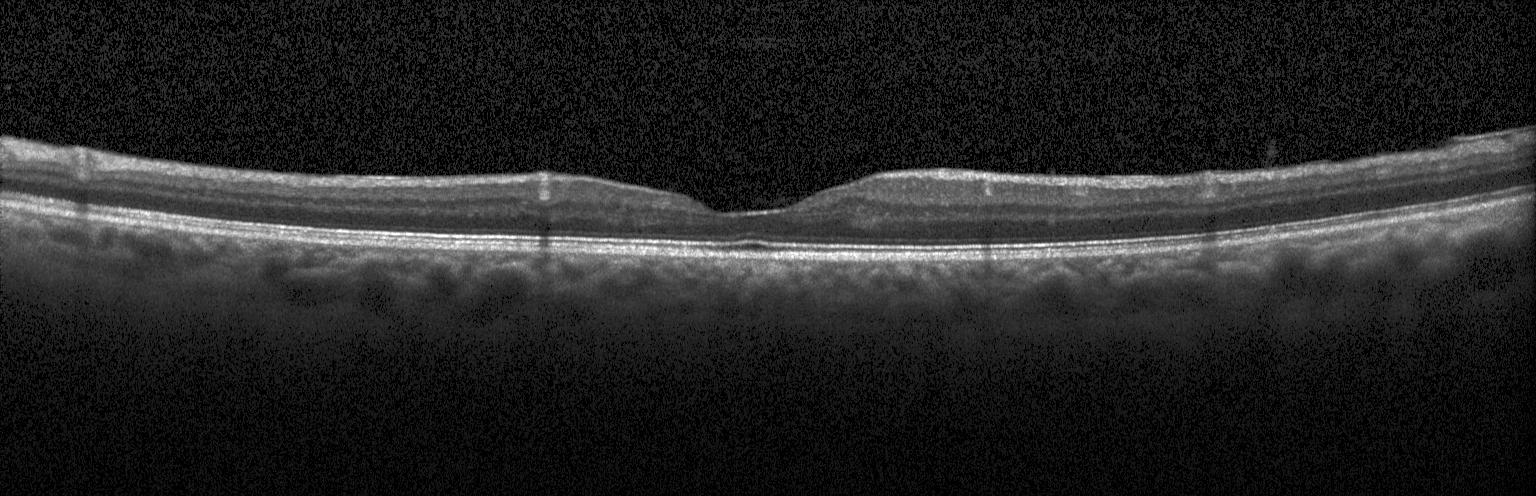 Diagnosis: neither CNV, DME, nor drusen.